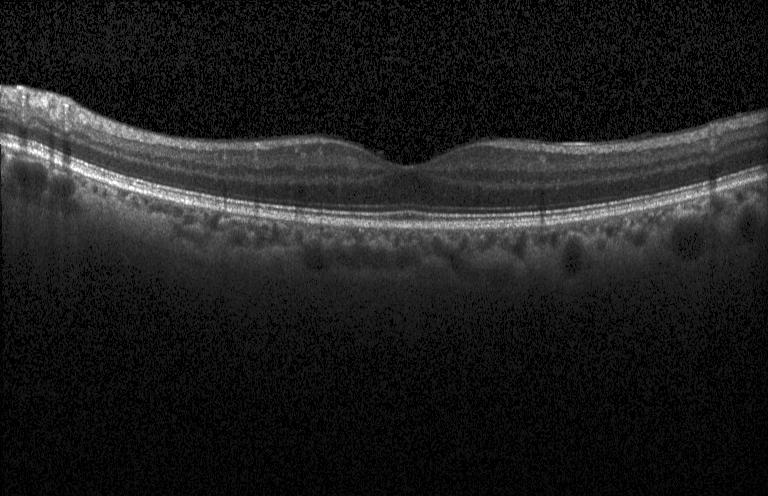

Spectral-domain OCT; acquired on a Heidelberg Spectralis; OCT B-scan; horizontal scan through the fovea.
No CNV, DME, or drusen.